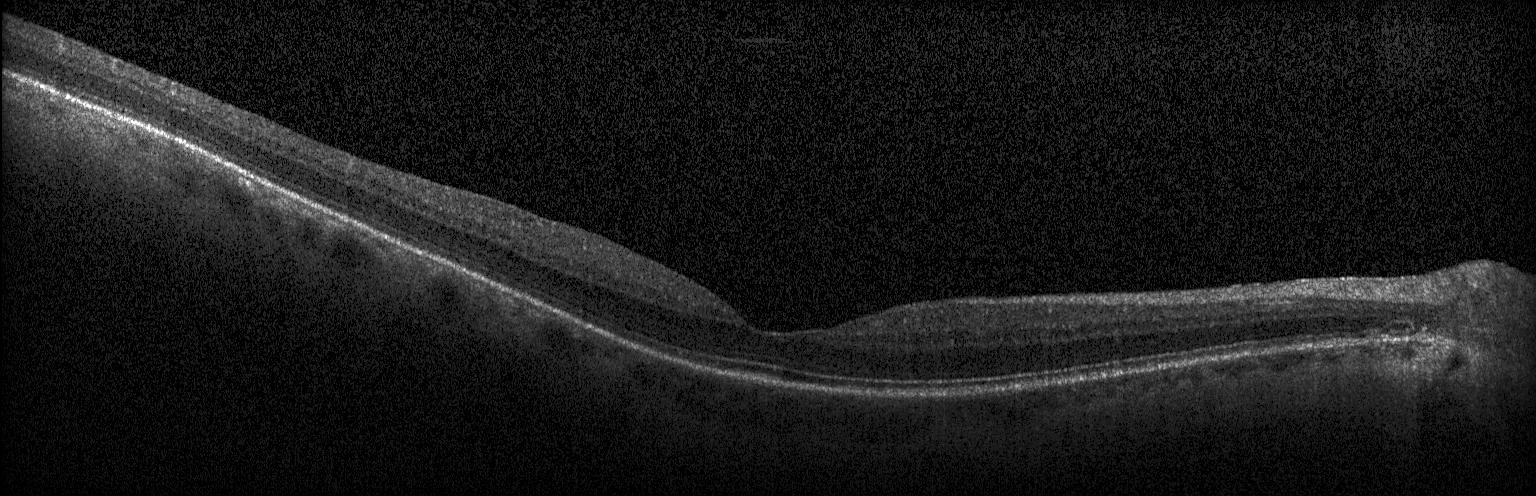
OCT B-scan showing no choroidal neovascularization, no diabetic macular edema, and no drusen.